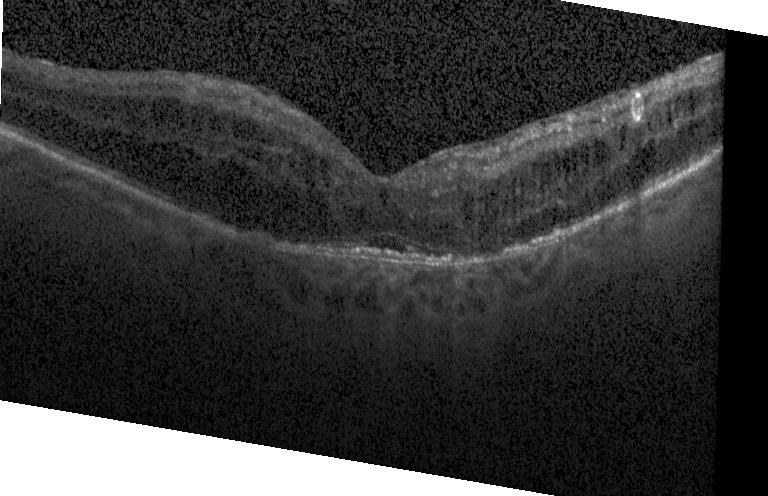

Retinal OCT B-scan. Centered on the fovea.
This B-scan demonstrates CNV.